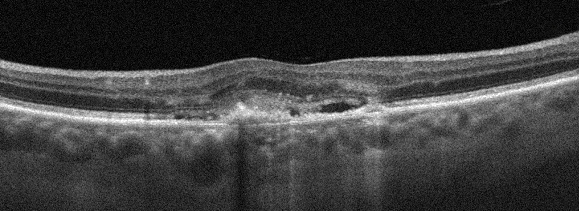

OD, macular scan, acquired on an Optovue Avanti RTVue XR, OCT line scan — OCT finding: age-related macular degeneration.